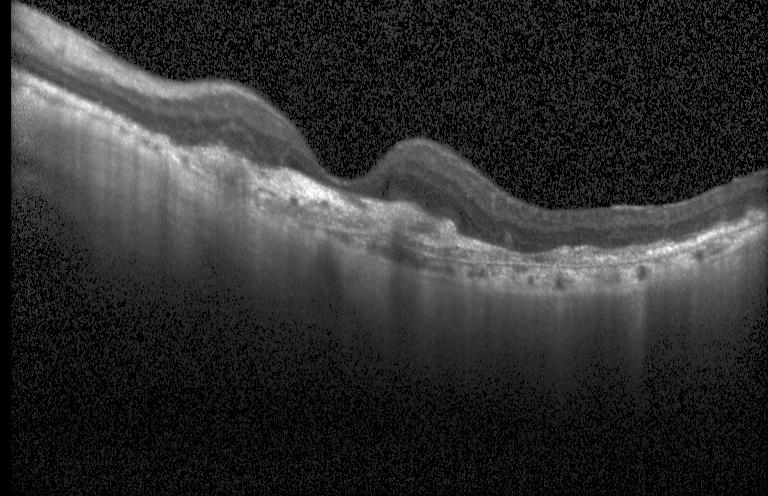
Finding: a choroidal neovascular membrane.